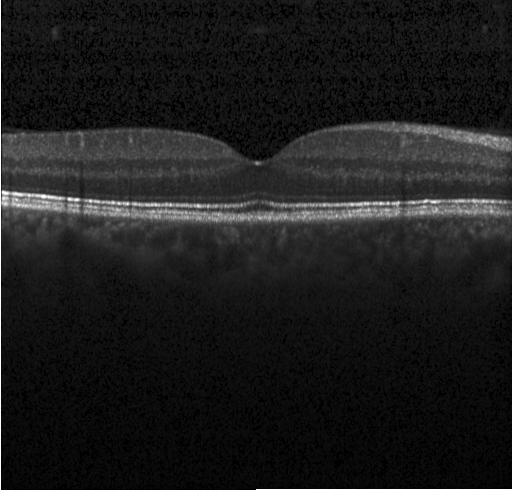

Spectral-domain optical coherence tomography · fovea-centered · optical coherence tomography scan — This B-scan demonstrates no choroidal neovascularization, diabetic macular edema, or drusen.